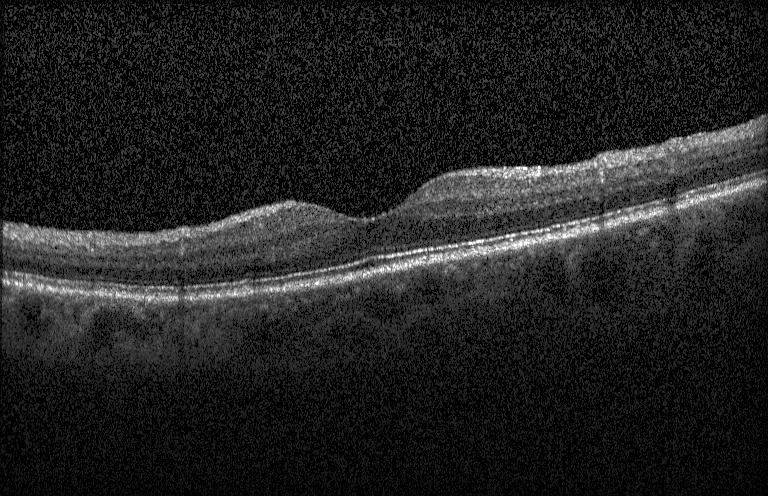
Fovea-centered. SD-OCT. Heidelberg Spectralis OCT system. Retinal OCT B-scan
Dx: no evidence of choroidal neovascularization, diabetic macular edema, or drusen.